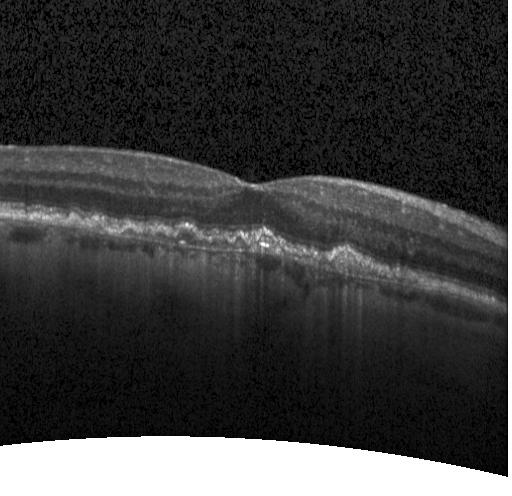

Heidelberg Spectralis OCT system · optical coherence tomography B-scan · spectral-domain OCT. A choroidal neovascular membrane.